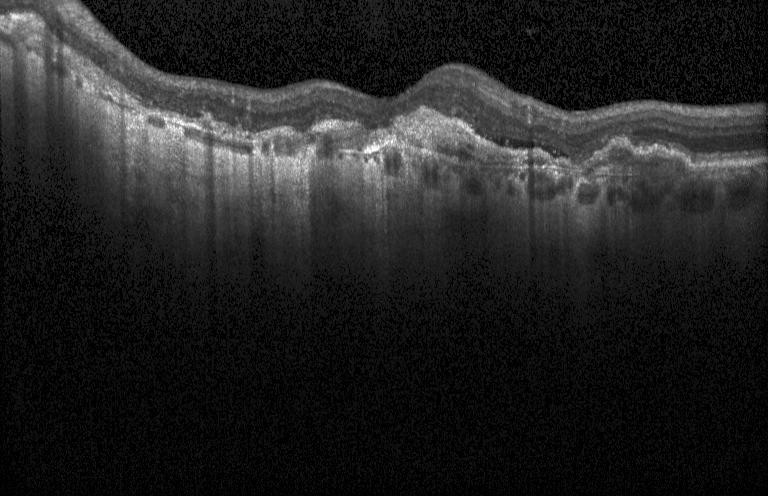

Diagnosis: choroidal neovascularization.